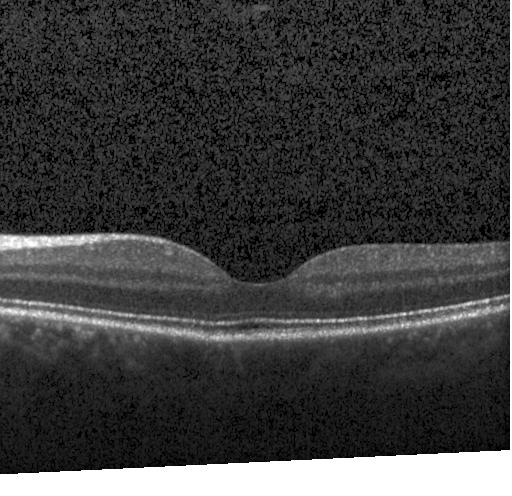 Macular OCT: no evidence of choroidal neovascularization, diabetic macular edema, or drusen.